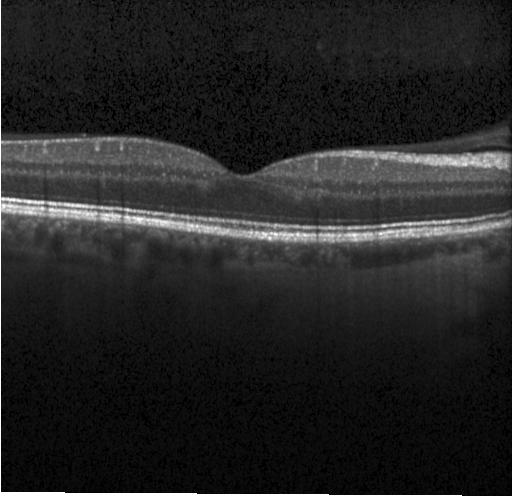
Optical coherence tomography B-scan, SD-OCT, through the macula, Heidelberg Spectralis OCT system. Diagnosis: no choroidal neovascularization, no diabetic macular edema, and no drusen.